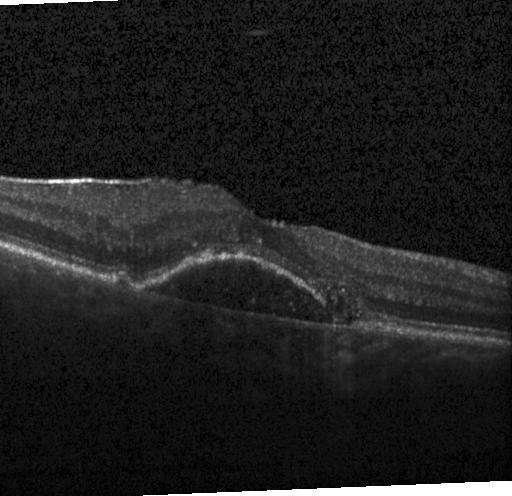 OCT finding: CNV.